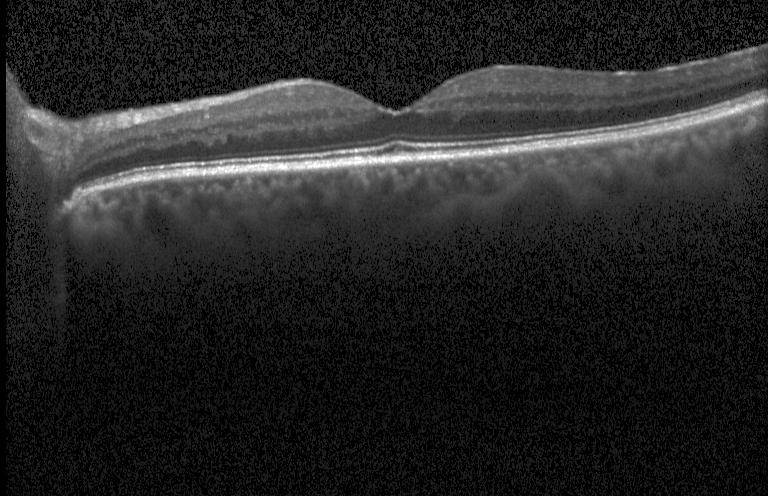

Optical coherence tomography B-scan · SD-OCT. Dx: neither choroidal neovascularization, diabetic macular edema, nor drusen.